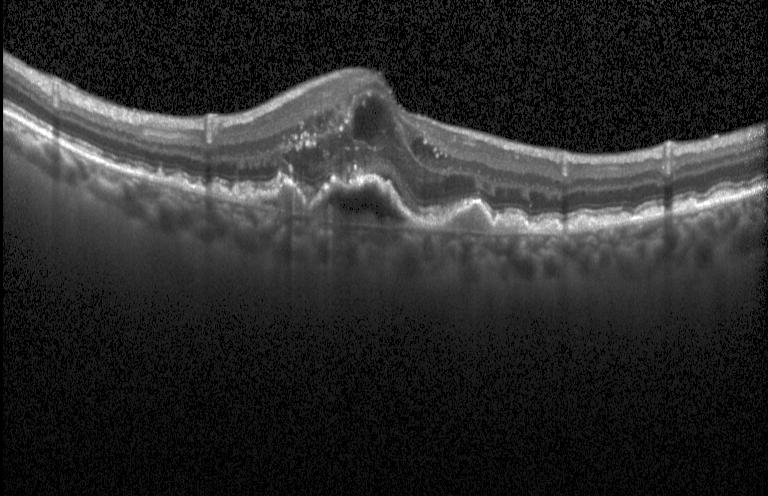

Acquired on a Heidelberg Spectralis · macular scan · retinal OCT cross-section.
Diagnosis: CNV.